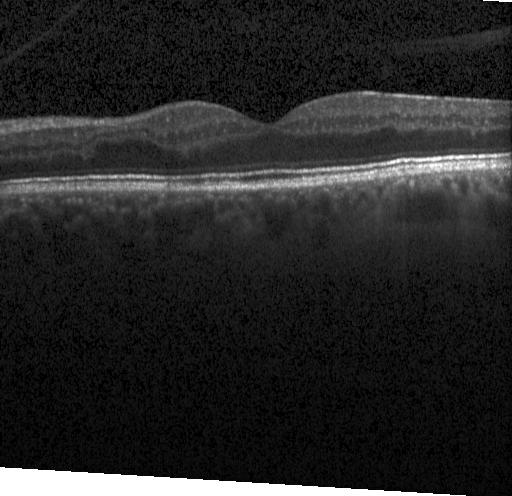

Impression: no choroidal neovascularization, diabetic macular edema, or drusen.